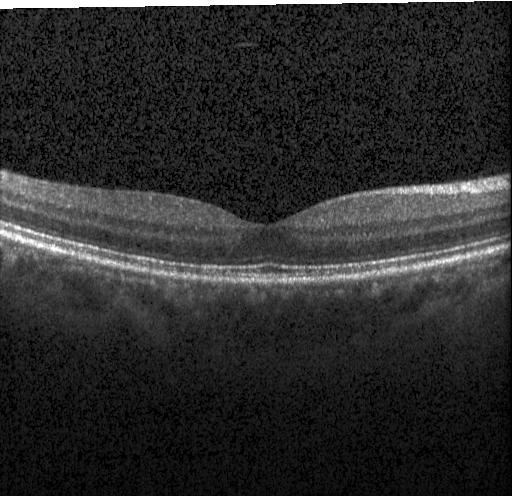
OCT scan showing no evidence of choroidal neovascularization, diabetic macular edema, or drusen.